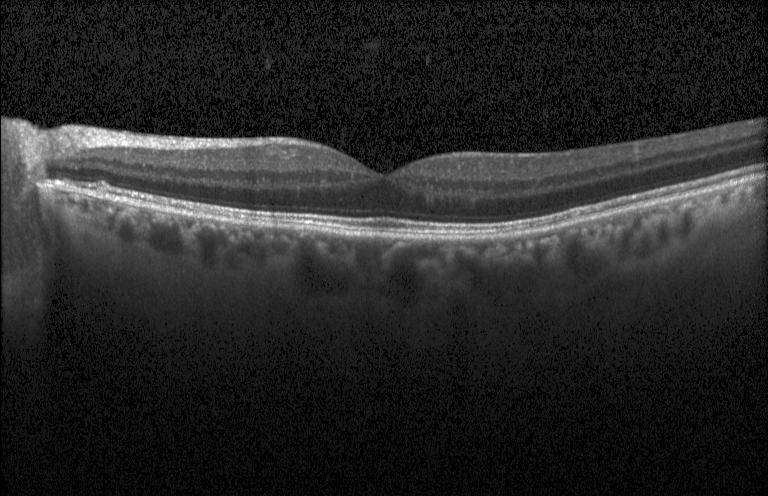
OCT line scan. Multiple drusen.